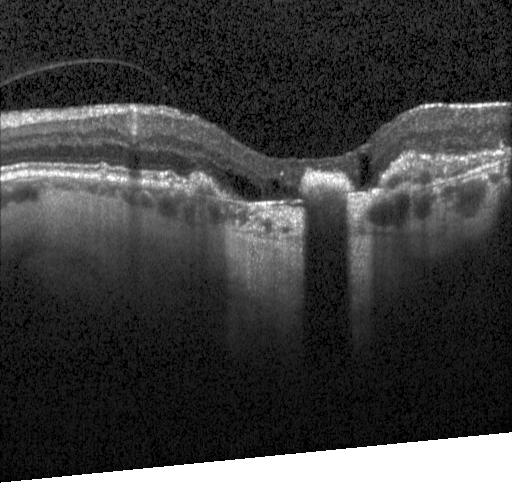
Dx: CNV.